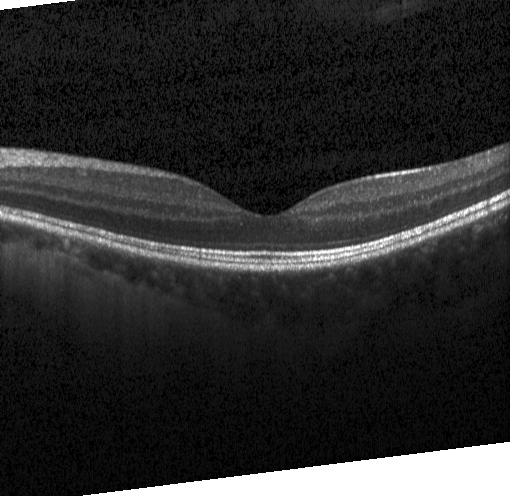

Heidelberg Spectralis OCT system. OCT B-scan. Horizontal scan through the fovea. Spectral-domain OCT.
Diagnosis: no evidence of choroidal neovascularization, diabetic macular edema, or drusen.